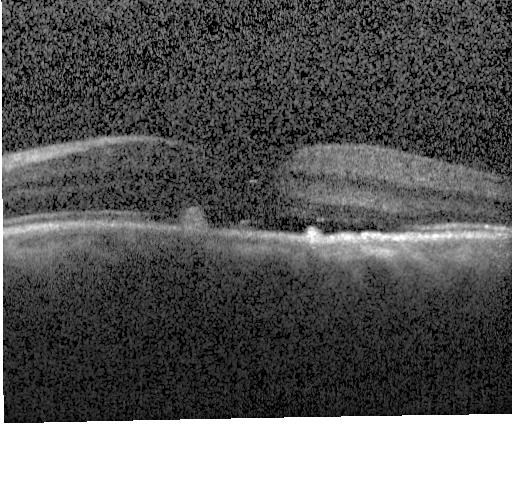

Acquired on a Heidelberg Spectralis; SD-OCT; optical coherence tomography scan.
Diagnosis: CNV.